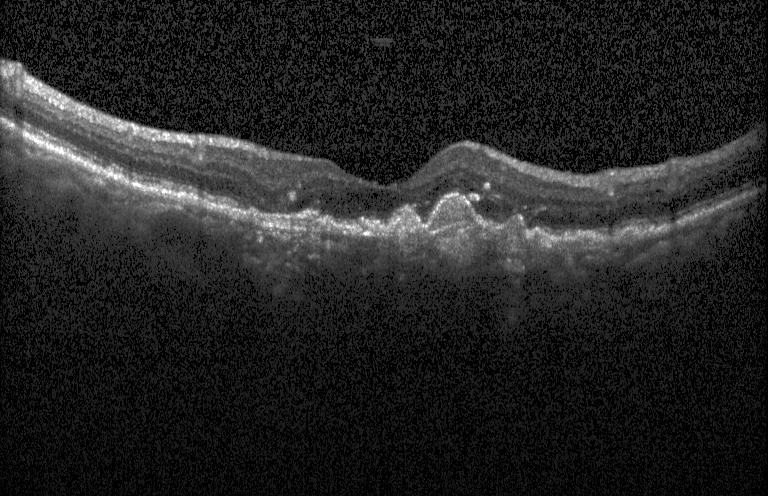
Optical coherence tomography scan — Diagnosis: choroidal neovascularization (CNV).